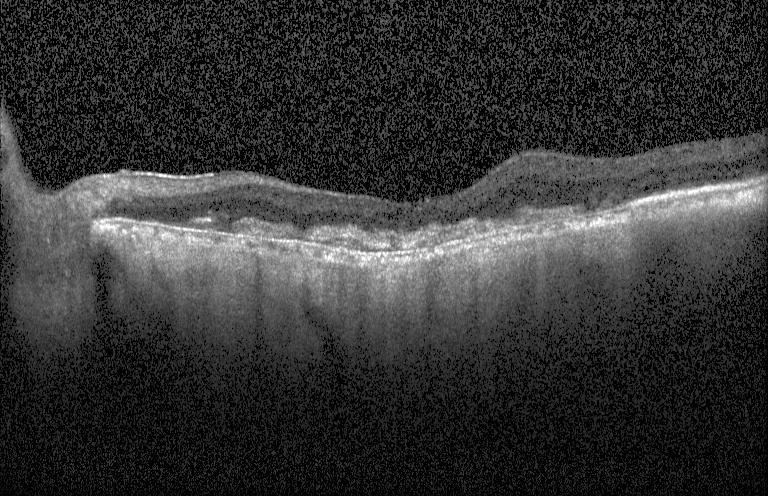
Optical coherence tomography B-scan. Through the macula.
Macular OCT: choroidal neovascularization.